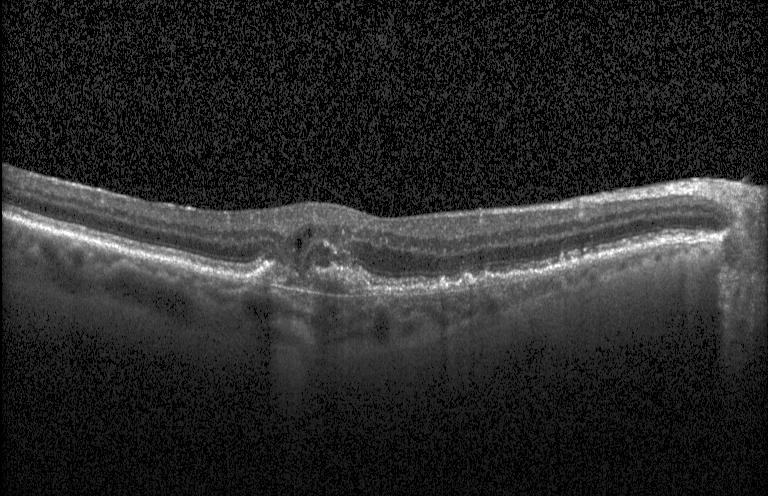

Spectral-domain optical coherence tomography, OCT B-scan.
A choroidal neovascular membrane.